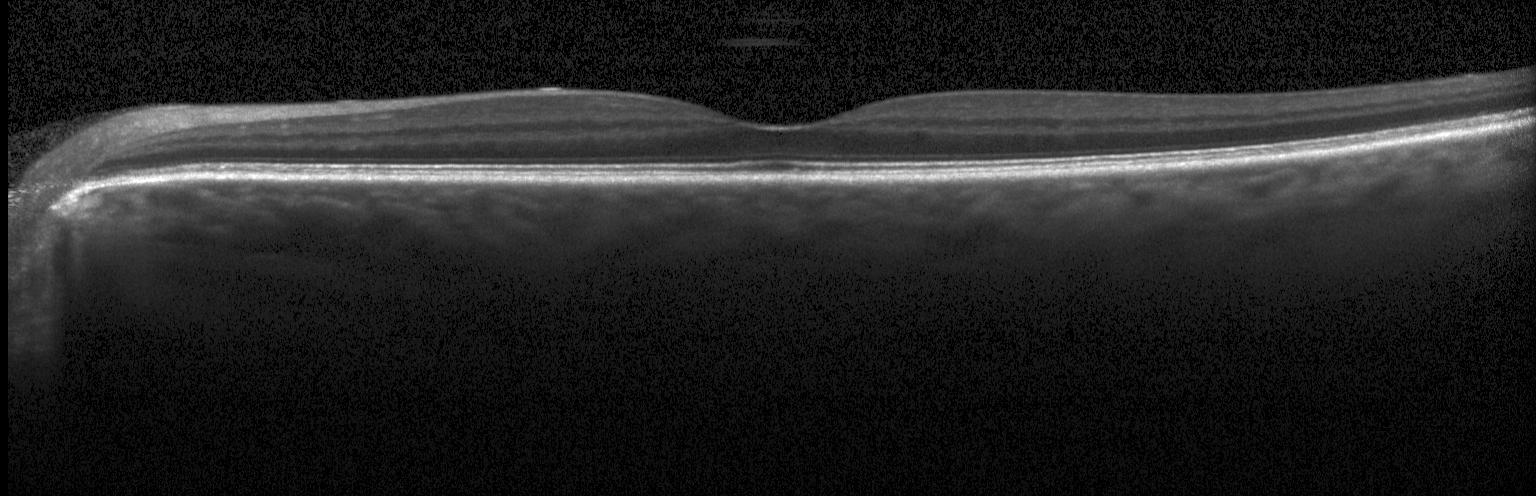
Macular scan; spectral-domain OCT; retinal OCT cross-section; Heidelberg Spectralis.
Diagnosis: no evidence of CNV, DME, or drusen.